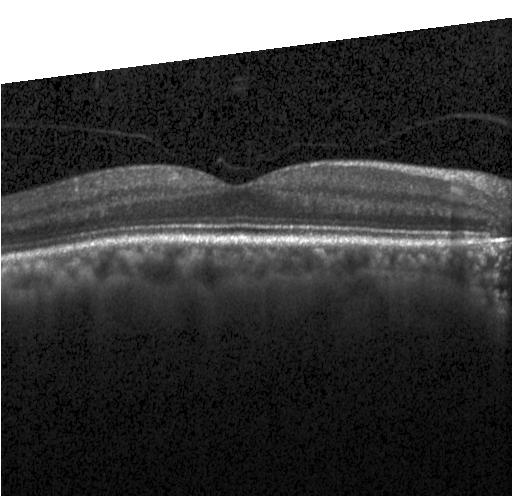
Spectral-domain optical coherence tomography, optical coherence tomography scan, acquired on a Heidelberg Spectralis. Dx: no CNV, no DME, and no drusen.